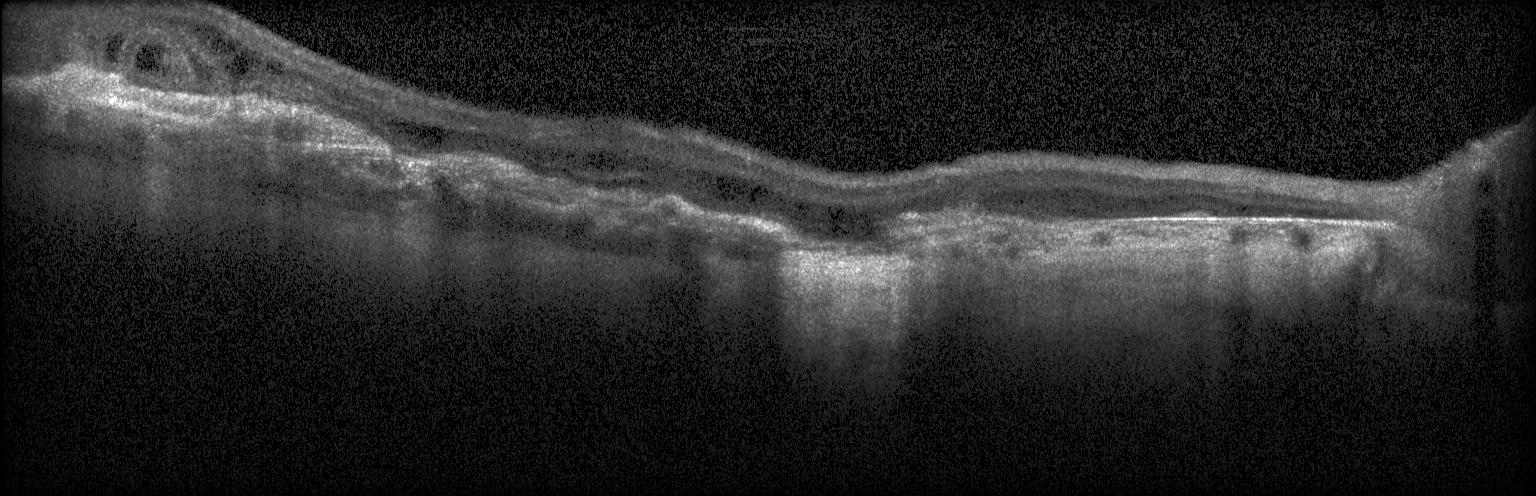

Heidelberg Spectralis OCT system; spectral-domain OCT; retinal OCT B-scan.
Impression: choroidal neovascularization.